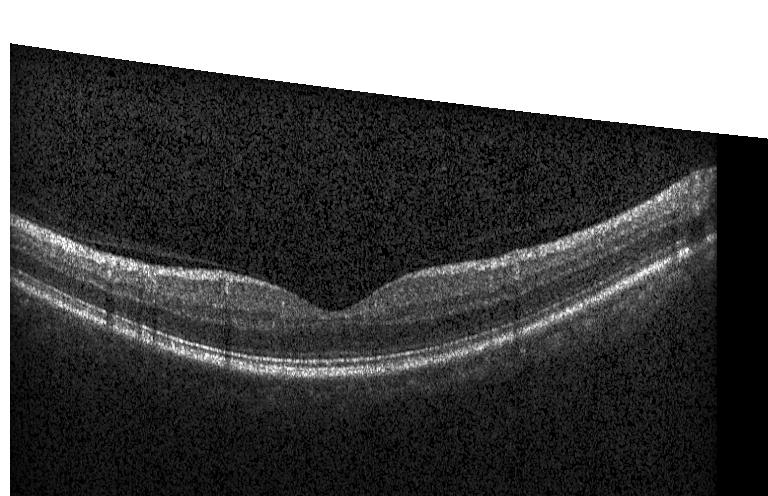
OCT scan showing no evidence of choroidal neovascularization, diabetic macular edema, or drusen.